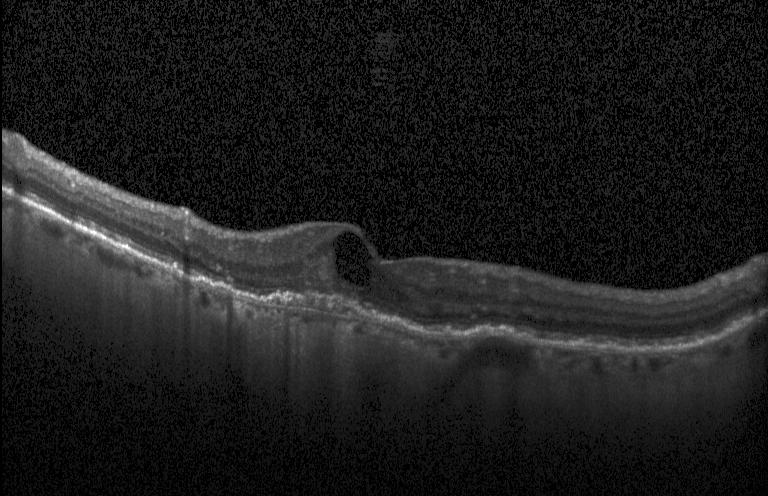 Spectral-domain OCT B-scan: choroidal neovascularization (CNV).